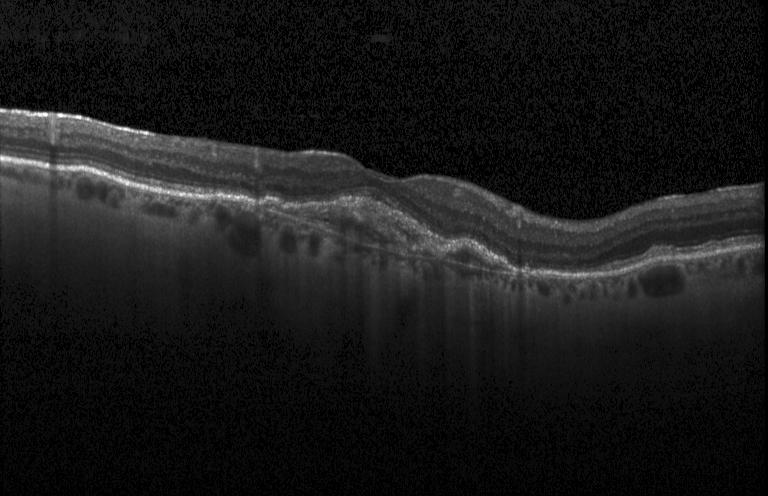
Optical coherence tomography scan; fovea-centered; acquired on a Heidelberg Spectralis; spectral-domain optical coherence tomography. This B-scan demonstrates choroidal neovascularization.